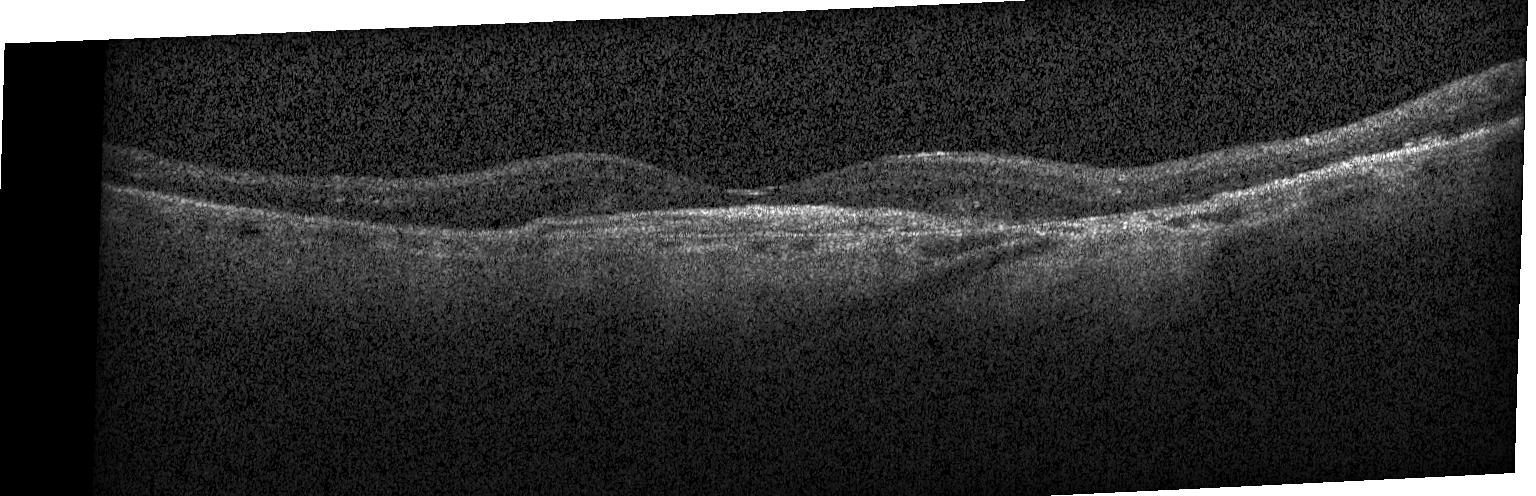
OCT scan showing a choroidal neovascular membrane.